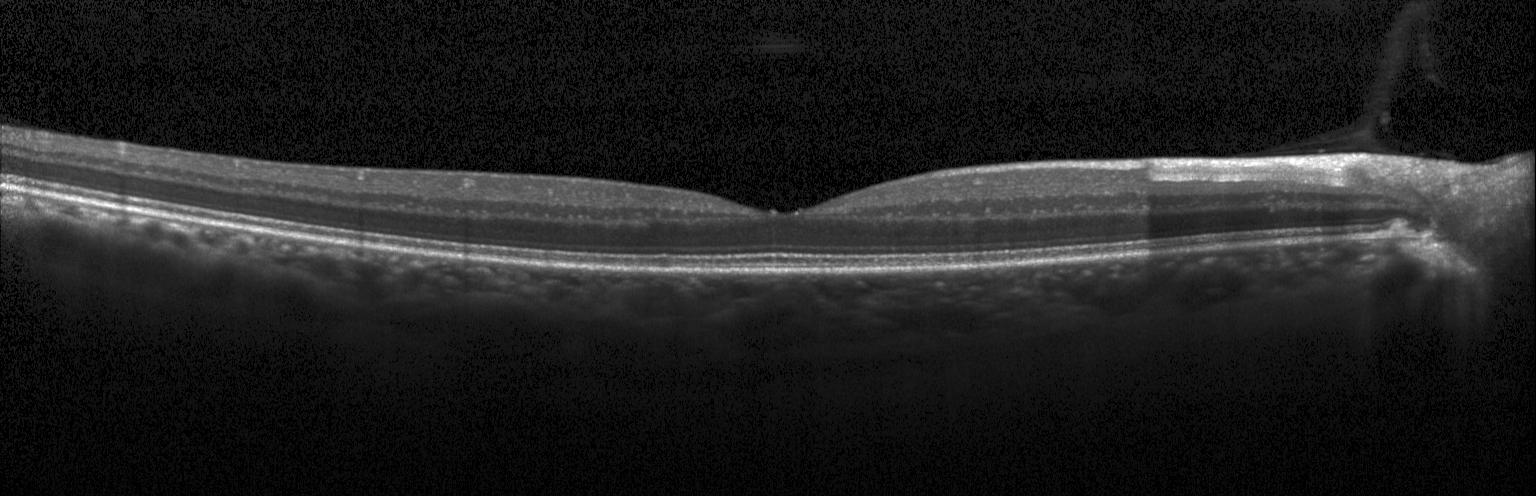
Retinal OCT cross-section, spectral-domain optical coherence tomography, macular scan.
Finding: neither CNV, DME, nor drusen.